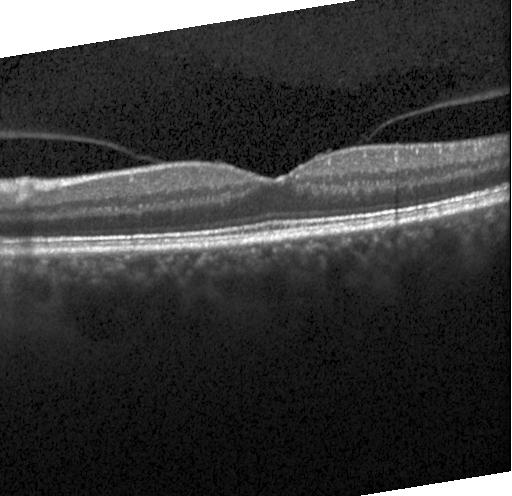

Fovea-centered · retinal OCT B-scan — Impression: no CNV, no DME, and no drusen.